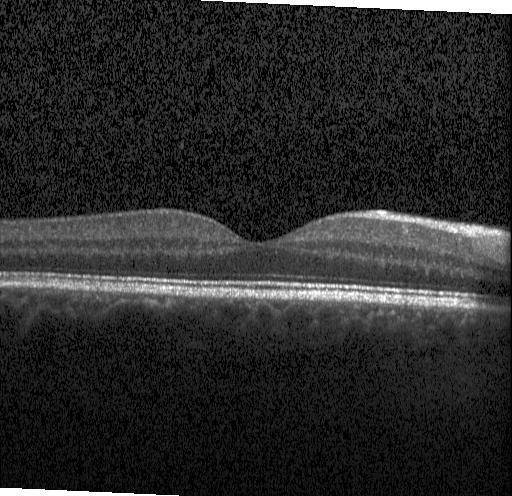
Retinal OCT cross-section. SD-OCT
Diagnosis: no choroidal neovascularization, diabetic macular edema, or drusen.